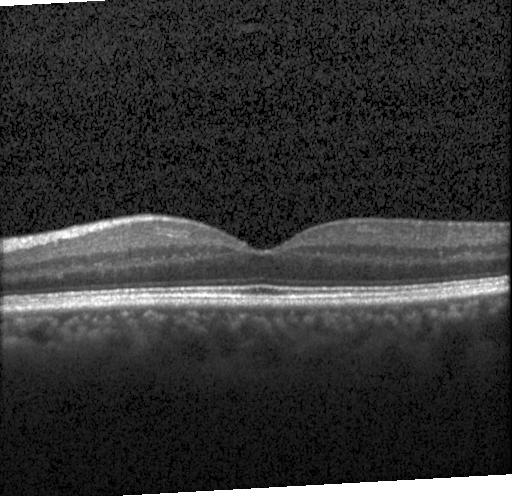 Retinal OCT cross-section showing neither CNV, DME, nor drusen.